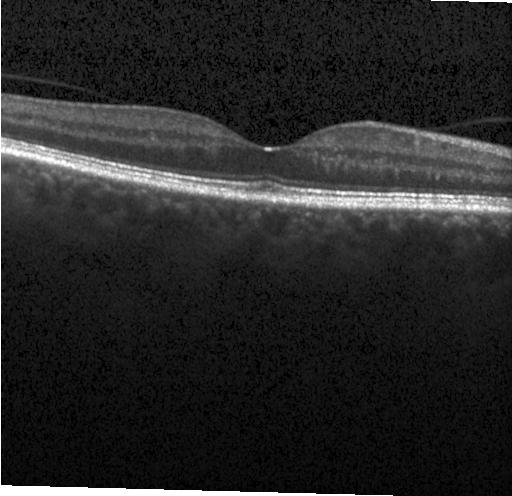

OCT B-scan showing no choroidal neovascularization, diabetic macular edema, or drusen.